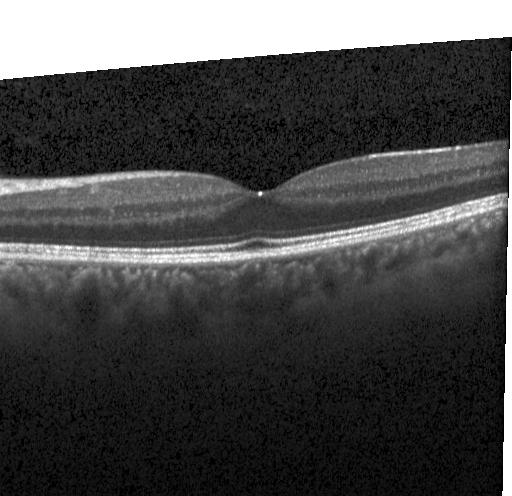

Optical coherence tomography scan; fovea-centered. OCT finding: neither CNV, DME, nor drusen.